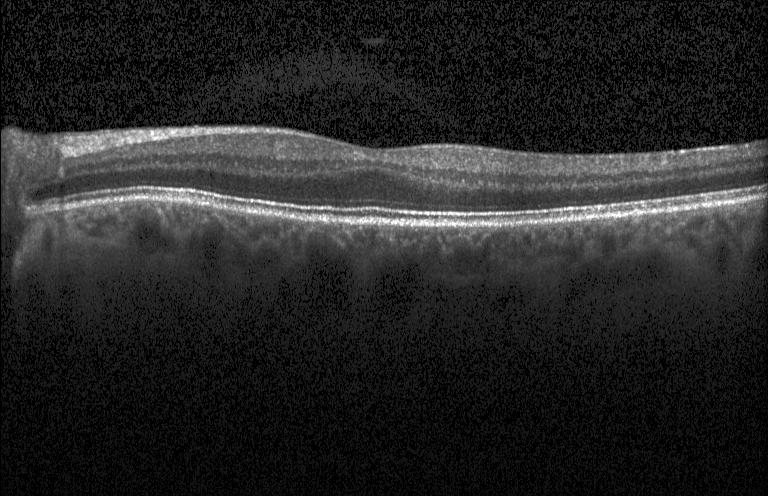 Instrument: Heidelberg Spectralis · spectral-domain optical coherence tomography · retinal OCT B-scan · centered on the fovea
Finding: no choroidal neovascularization, no diabetic macular edema, and no drusen.